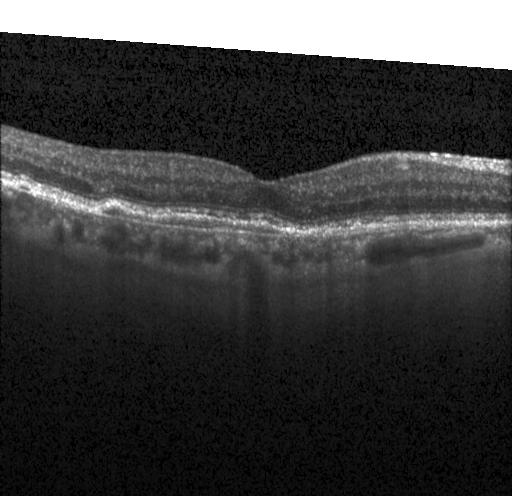 Retinal OCT cross-section showing choroidal neovascularization.